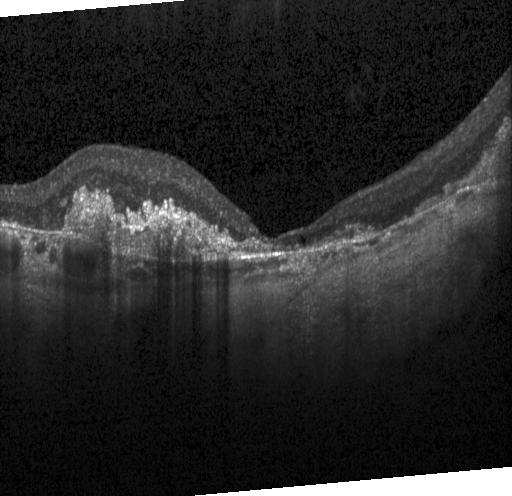 Macular scan; retinal OCT cross-section. This B-scan demonstrates a choroidal neovascular membrane.